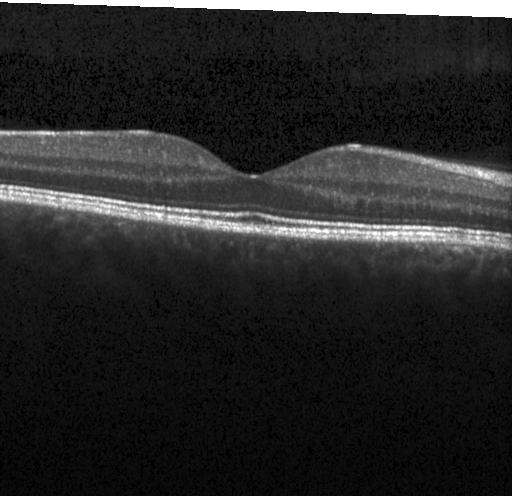 Through the macula; instrument: Heidelberg Spectralis; optical coherence tomography B-scan. Finding: no choroidal neovascularization, no diabetic macular edema, and no drusen.